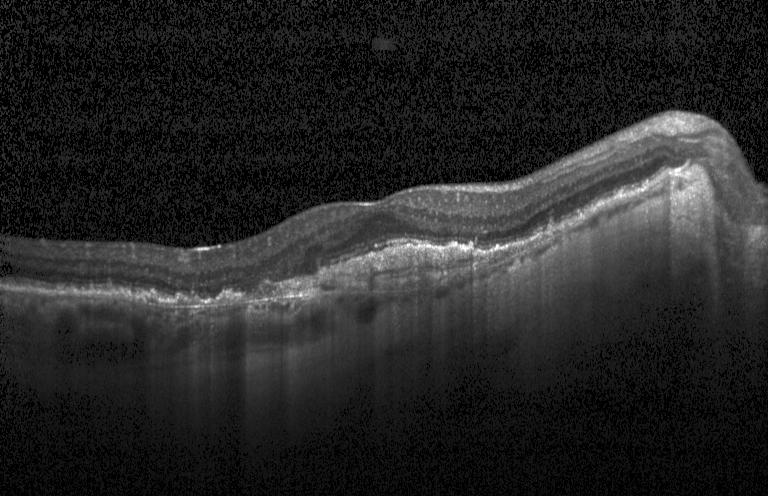
Centered on the fovea. Acquired on a Heidelberg Spectralis. OCT B-scan. Macular OCT: choroidal neovascularization (CNV).